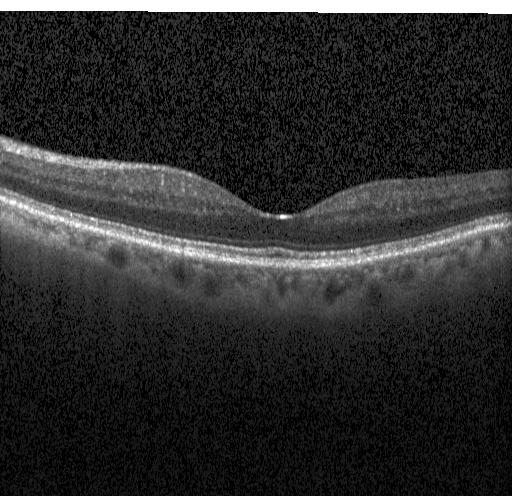 Macular OCT demonstrating no choroidal neovascularization, no diabetic macular edema, and no drusen.